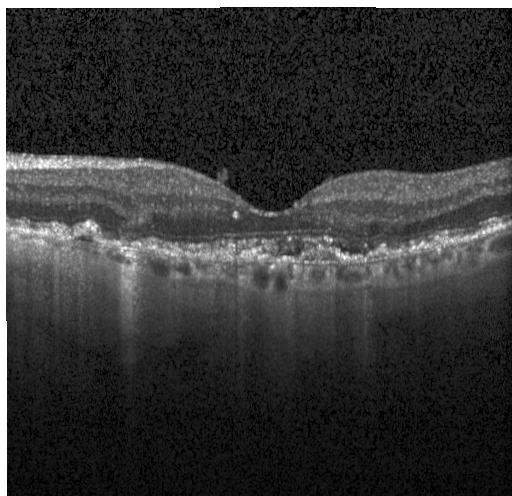 Impression: choroidal neovascularization (CNV).